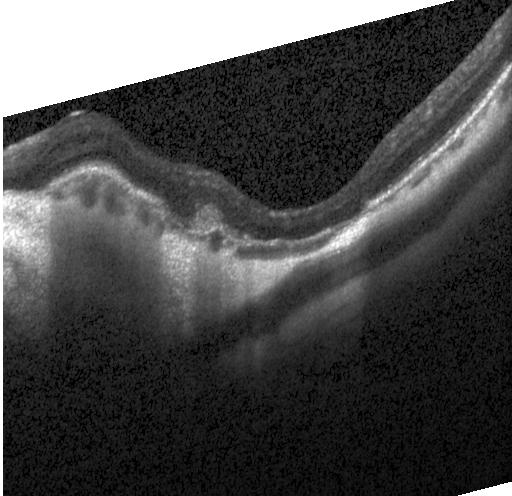

Retinal OCT cross-section showing choroidal neovascularization.